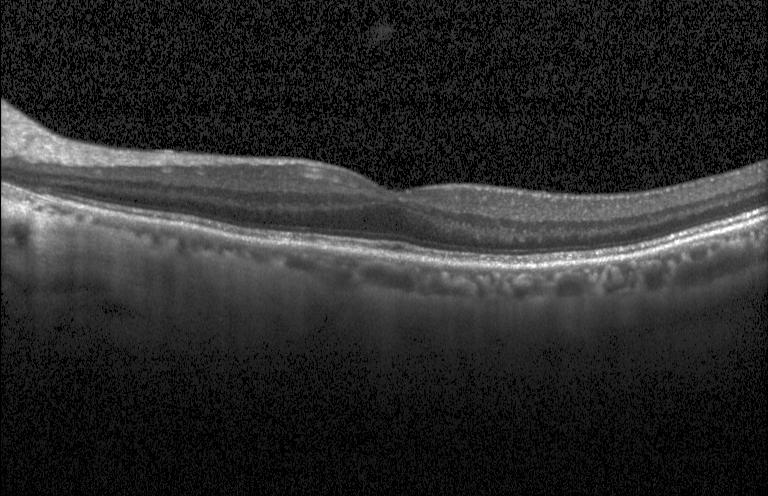 Optical coherence tomography scan. This B-scan demonstrates neither CNV, DME, nor drusen.